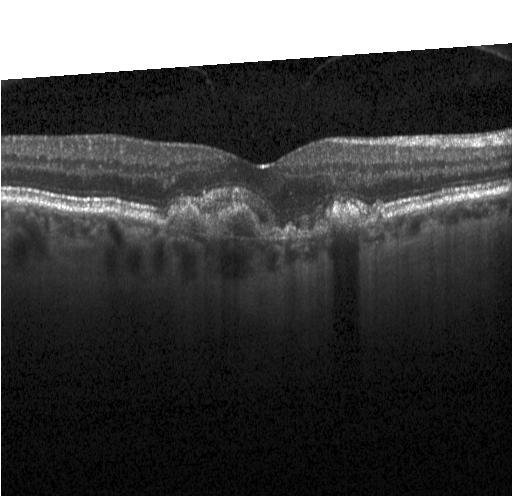
Retinal OCT B-scan.
Finding: choroidal neovascularization (CNV).